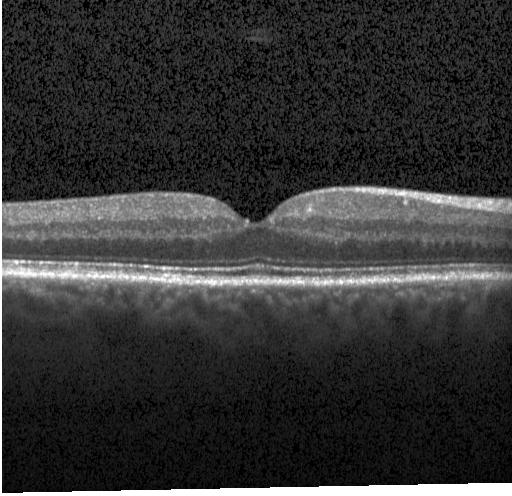

Acquired on a Heidelberg Spectralis. Centered on the fovea. Spectral-domain OCT. Retinal OCT cross-section. Impression: no choroidal neovascularization, diabetic macular edema, or drusen.